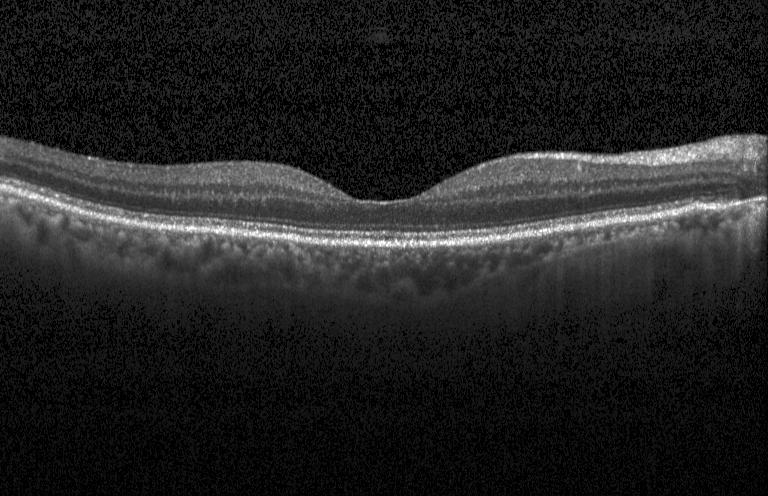 Impression: no choroidal neovascularization, no diabetic macular edema, and no drusen.